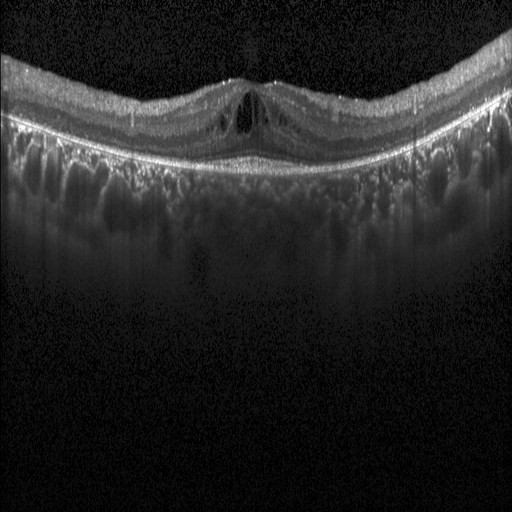
OCT scan showing diabetic macular edema (DME).